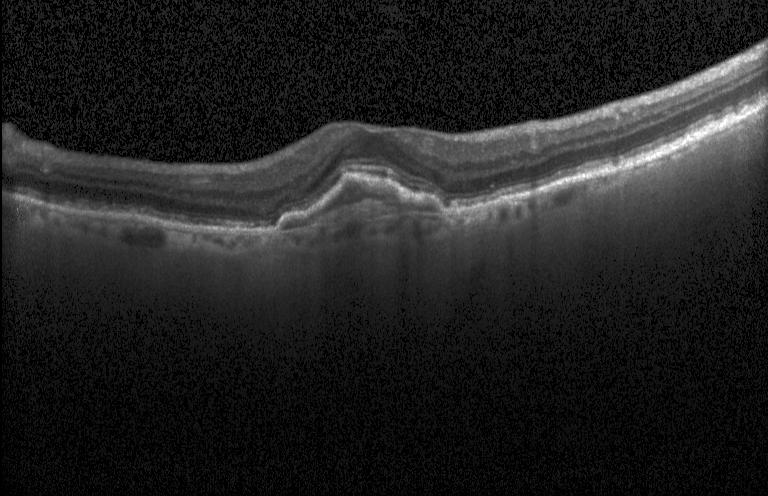
Spectral-domain OCT; Heidelberg Spectralis OCT system; retinal OCT cross-section. A choroidal neovascular membrane.